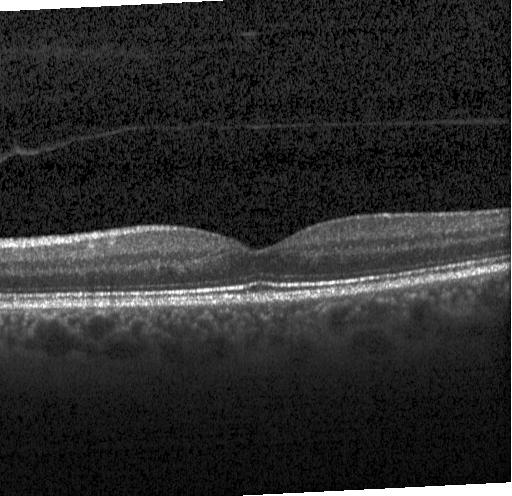
Fovea-centered, optical coherence tomography scan, Heidelberg Spectralis. No choroidal neovascularization, diabetic macular edema, or drusen.